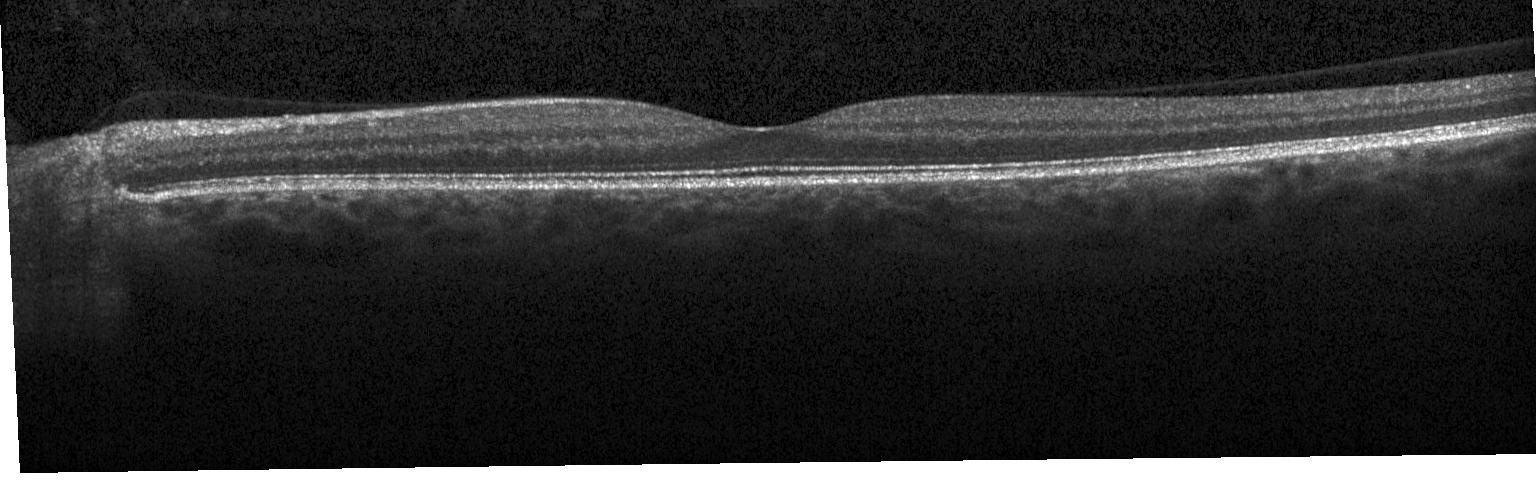

This B-scan demonstrates no choroidal neovascularization, no diabetic macular edema, and no drusen.